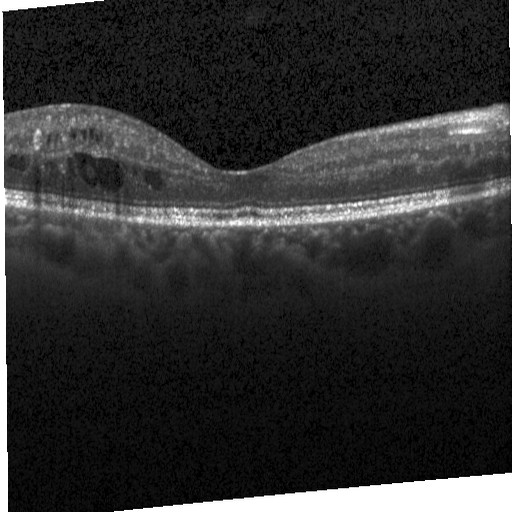 Retinal OCT cross-section. Finding: diabetic macular edema (DME).